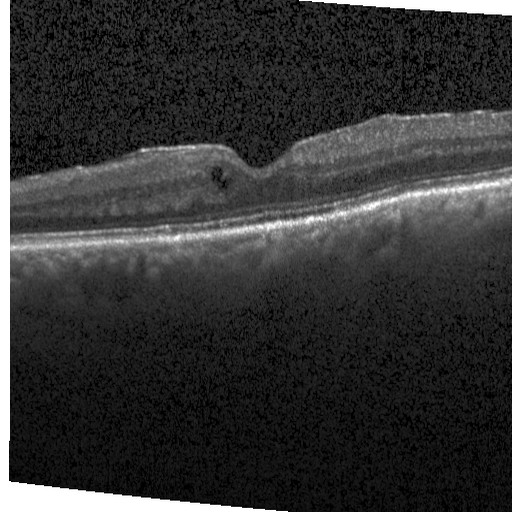
Impression: diabetic macular edema (DME).